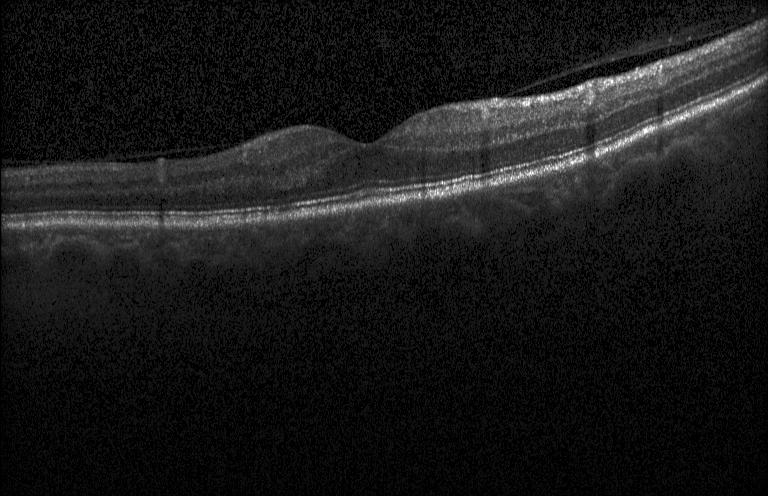

Spectral-domain optical coherence tomography · retinal OCT cross-section. Macular OCT: neither choroidal neovascularization, diabetic macular edema, nor drusen.